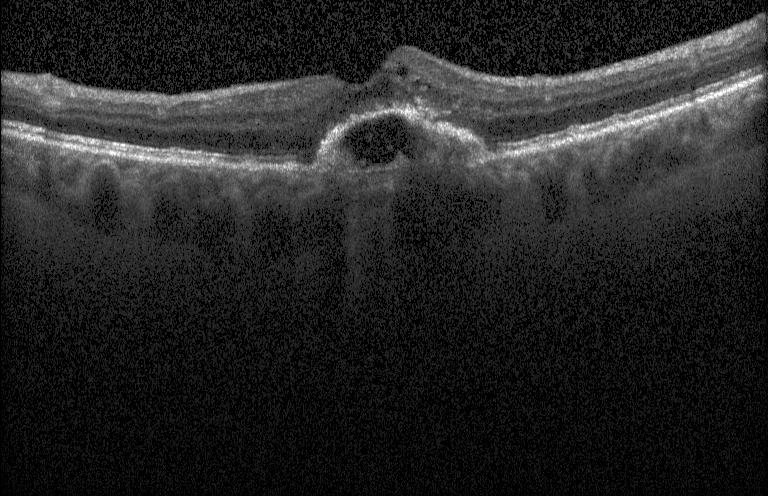

Optical coherence tomography scan · spectral-domain OCT
Finding: choroidal neovascularization.